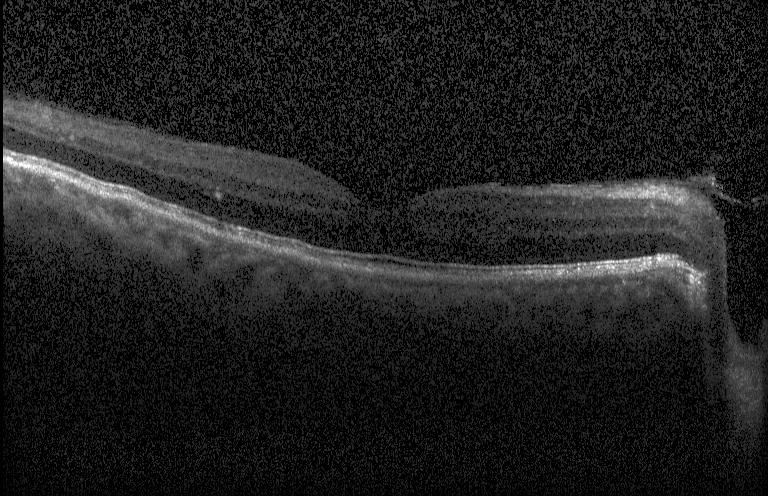

Heidelberg Spectralis, OCT B-scan, through the macula. Finding: neither choroidal neovascularization, diabetic macular edema, nor drusen.